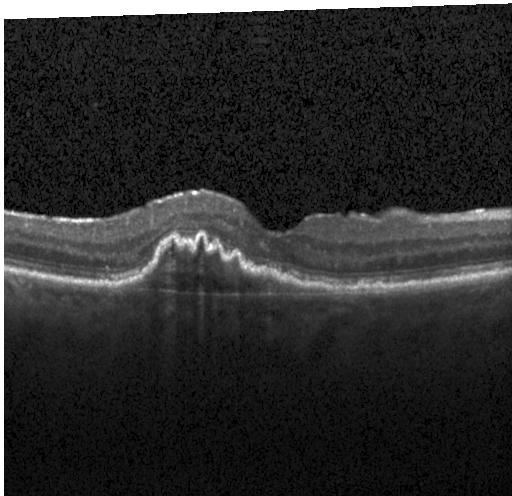
OCT B-scan; fovea-centered
Impression: CNV.